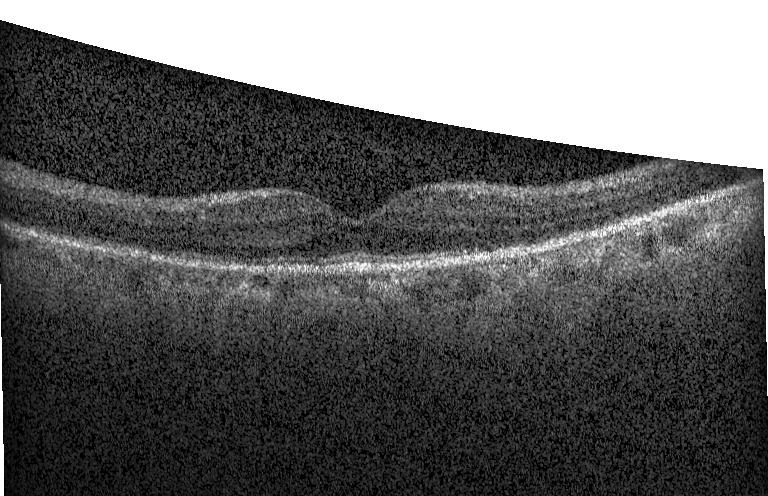
OCT line scan. Impression: no evidence of CNV, DME, or drusen.